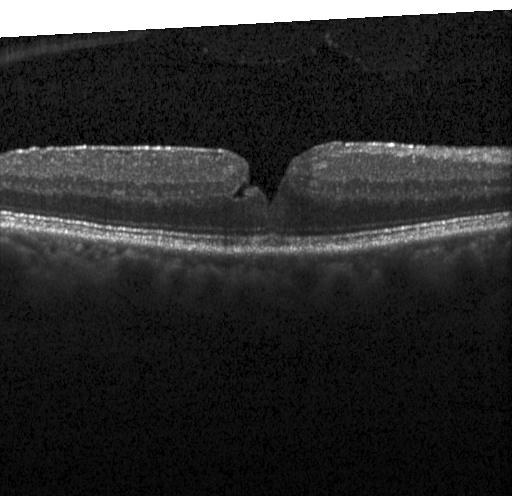

Spectral-domain OCT; retinal OCT cross-section
This B-scan demonstrates diabetic macular edema (DME).